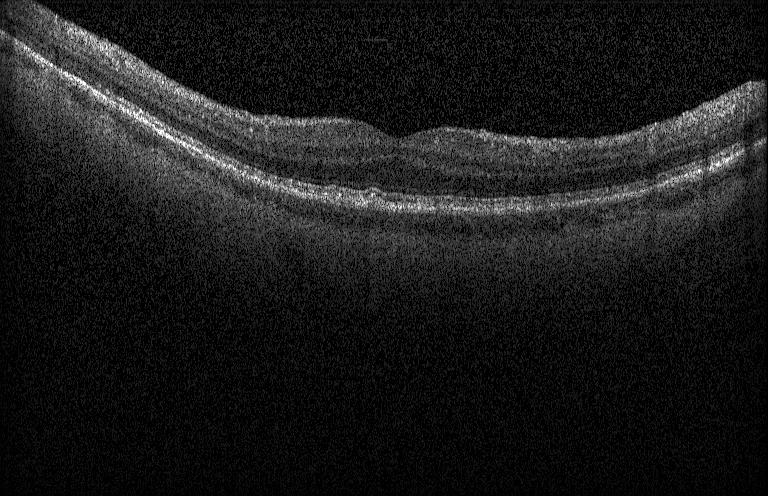 SD-OCT. Retinal OCT B-scan. Through the macula. OCT finding: multiple drusen.